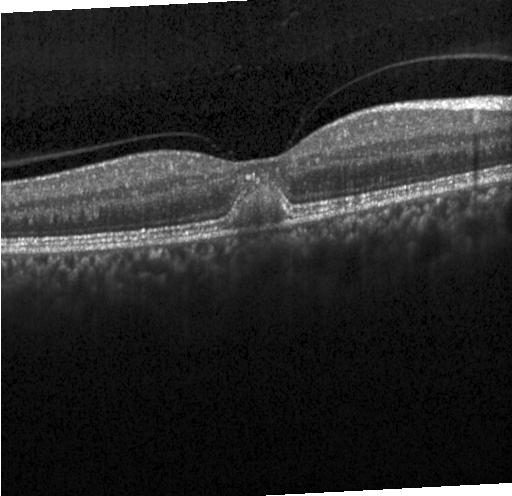
Retinal OCT cross-section
Assessment: a choroidal neovascular membrane.